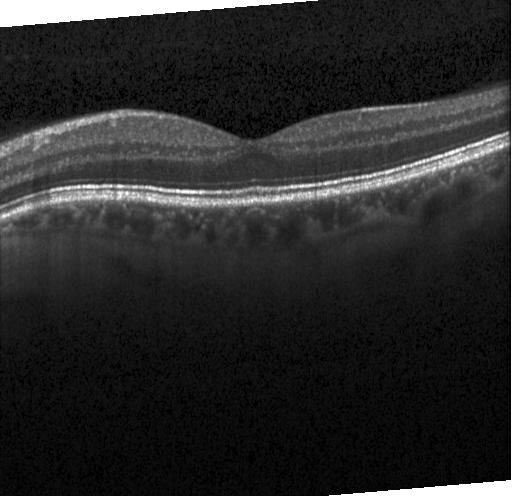
Optical coherence tomography scan, fovea-centered.
This B-scan demonstrates no choroidal neovascularization, diabetic macular edema, or drusen.